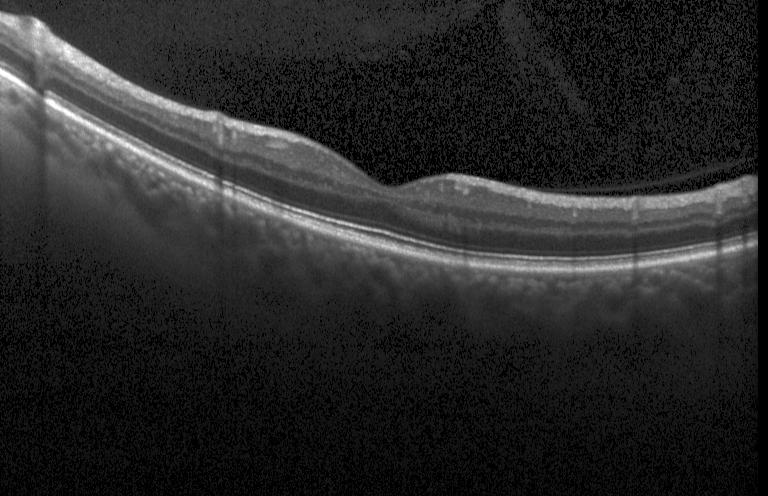

Acquired on a Heidelberg Spectralis, optical coherence tomography scan.
Diagnosis: no choroidal neovascularization, no diabetic macular edema, and no drusen.